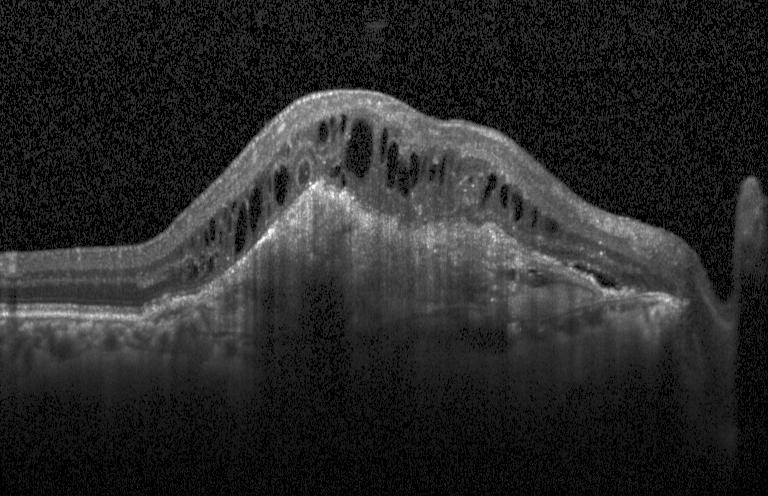
Heidelberg Spectralis OCT system · spectral-domain OCT · retinal OCT cross-section · fovea-centered. OCT finding: choroidal neovascularization.